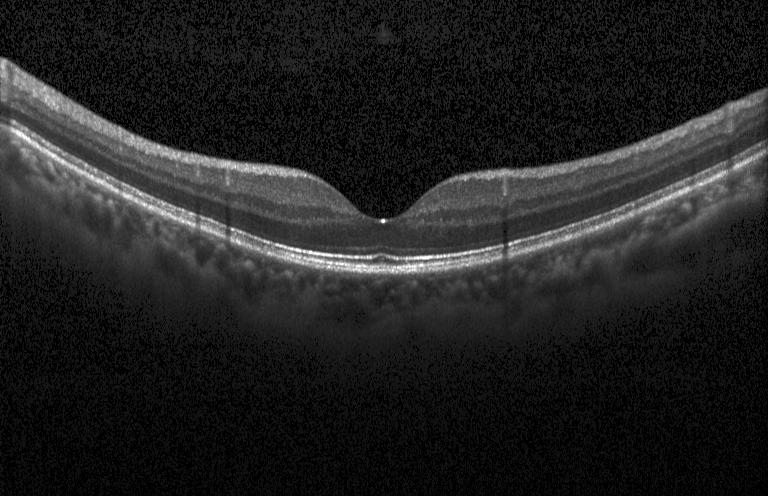 Finding: no evidence of choroidal neovascularization, diabetic macular edema, or drusen.